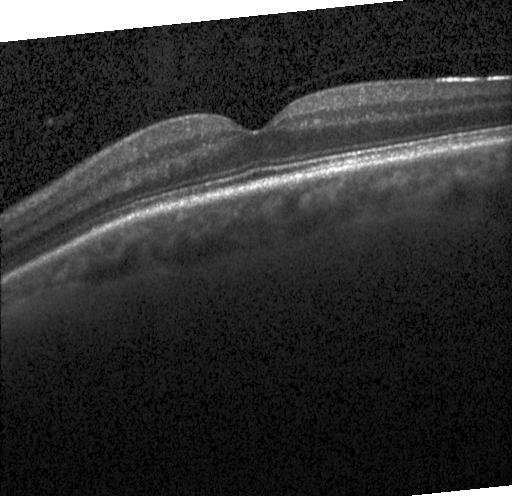

Optical coherence tomography B-scan
Assessment: no evidence of choroidal neovascularization, diabetic macular edema, or drusen.